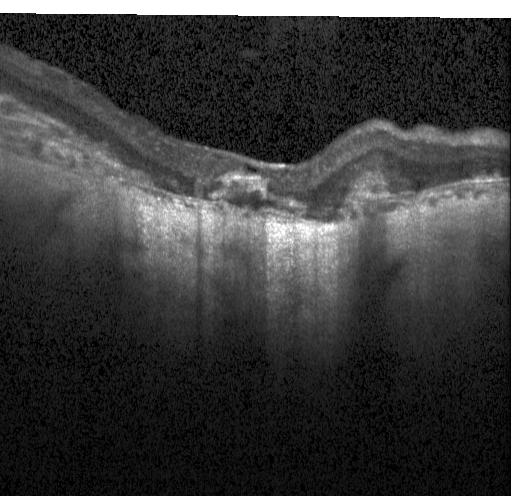

OCT B-scan showing a choroidal neovascular membrane.